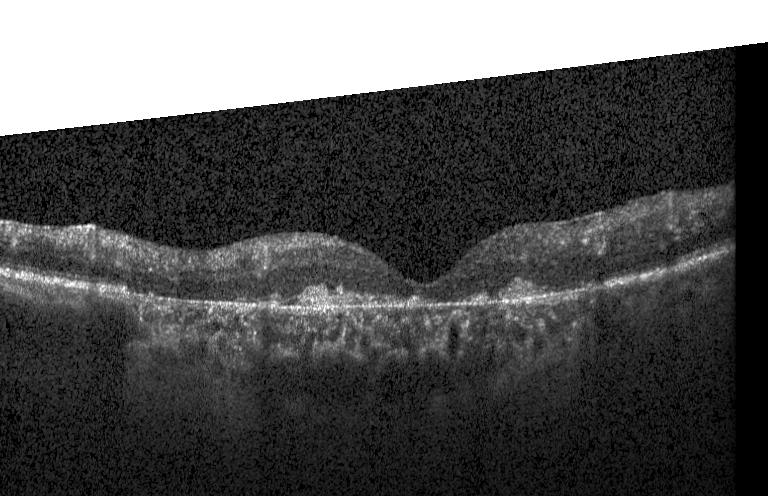

Heidelberg Spectralis; SD-OCT; horizontal scan through the fovea; retinal OCT cross-section — Finding: CNV.